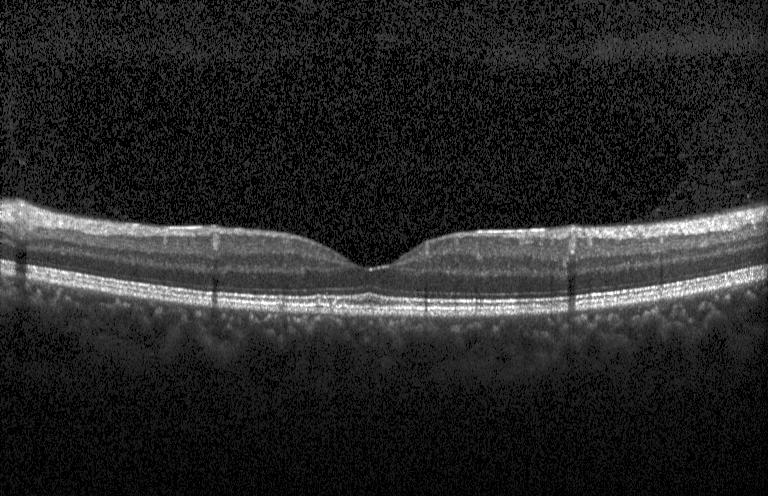

Retinal OCT cross-section showing no CNV, no DME, and no drusen.